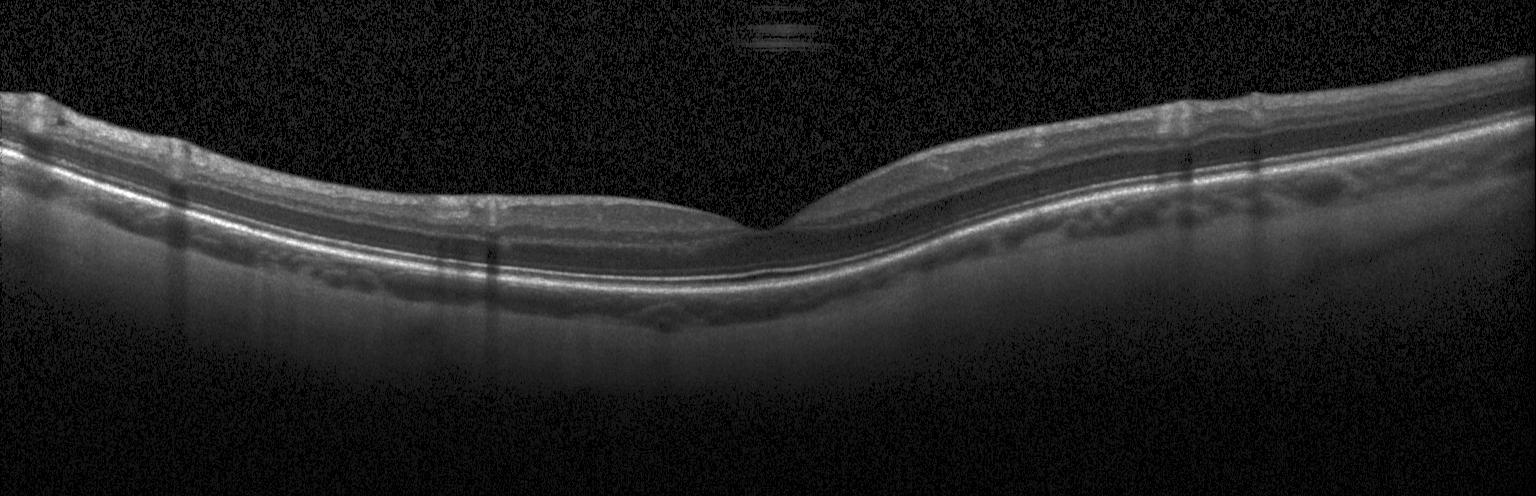

Macular OCT demonstrating no evidence of CNV, DME, or drusen.